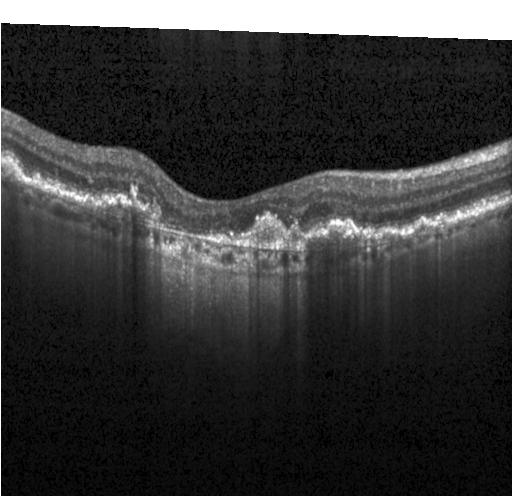 Impression: choroidal neovascularization (CNV).